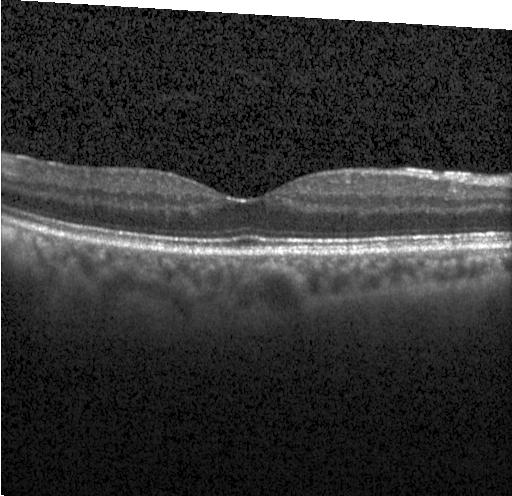
OCT B-scan showing neither CNV, DME, nor drusen.